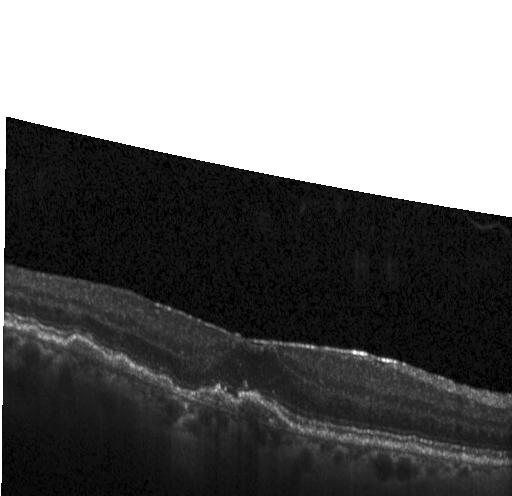 Macular OCT: a choroidal neovascular membrane.